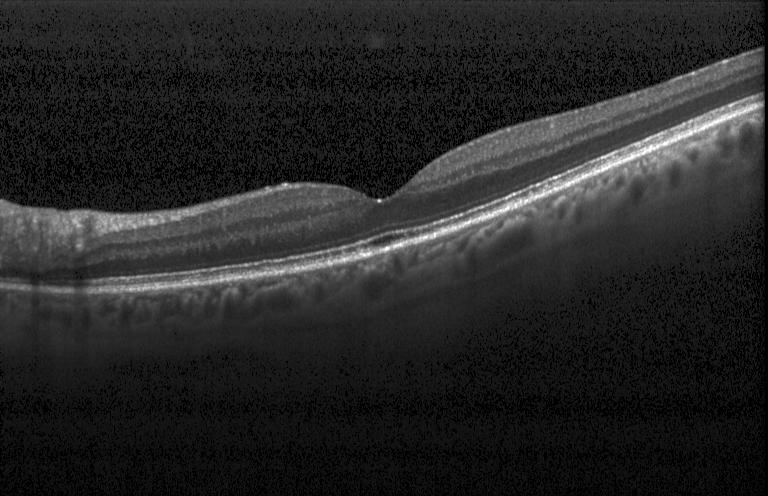

Spectral-domain optical coherence tomography; retinal OCT cross-section. Impression: no CNV, no DME, and no drusen.